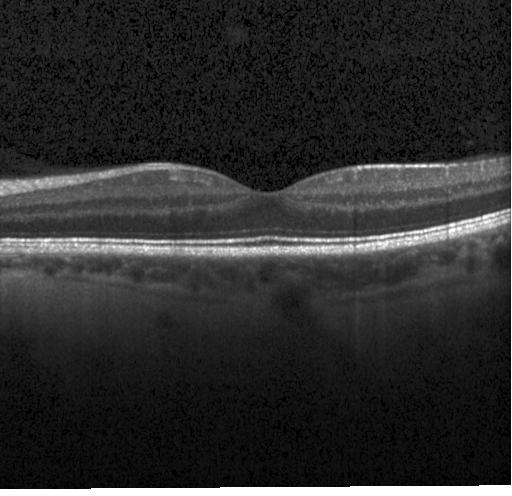

No evidence of CNV, DME, or drusen.